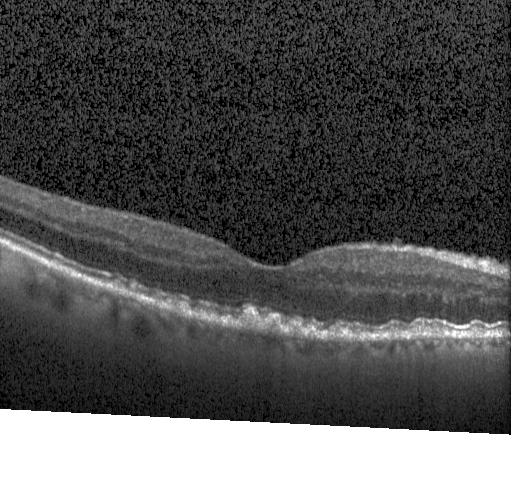
OCT finding: sub-RPE drusenoid deposits.